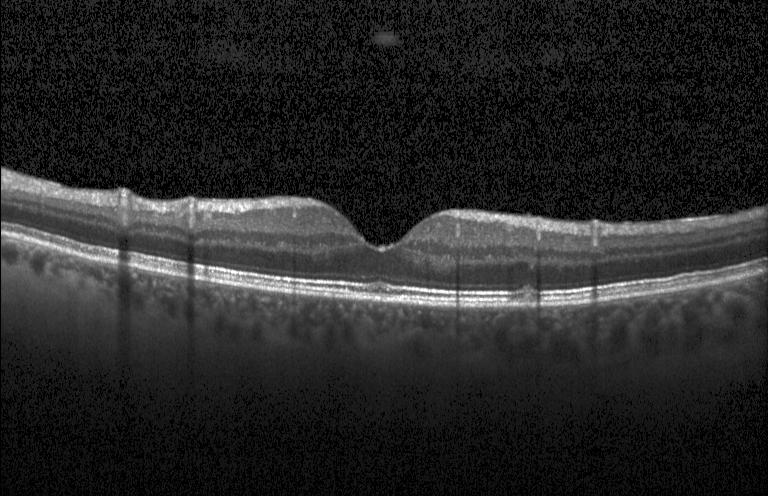

Retinal OCT B-scan; acquired on a Heidelberg Spectralis; horizontal scan through the fovea.
Impression: sub-RPE drusenoid deposits.